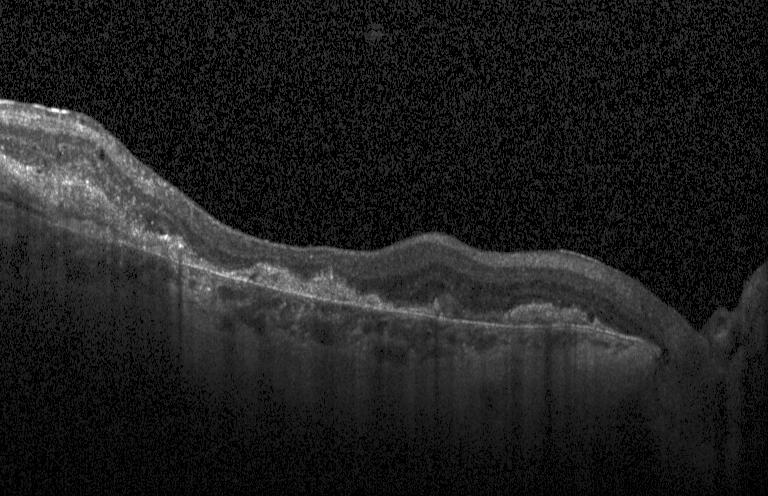
Retinal OCT B-scan. Diagnosis: a choroidal neovascular membrane.